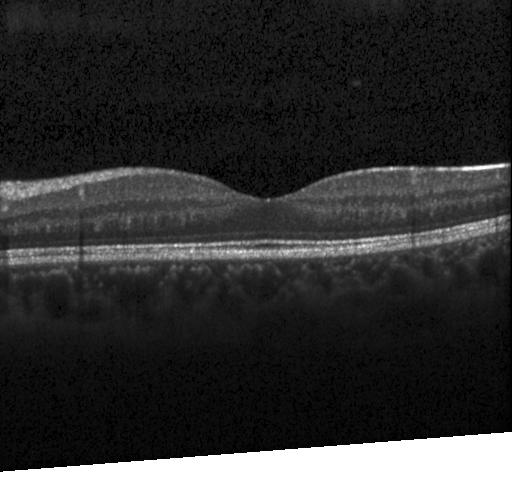 No choroidal neovascularization, no diabetic macular edema, and no drusen.